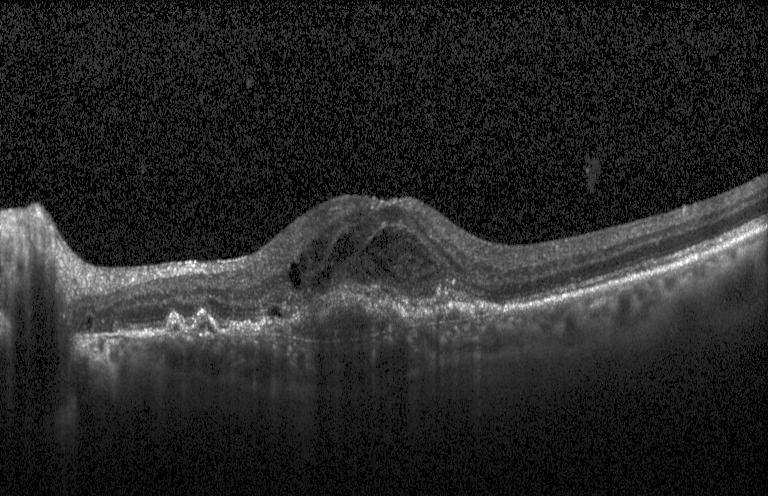 Dx: CNV.